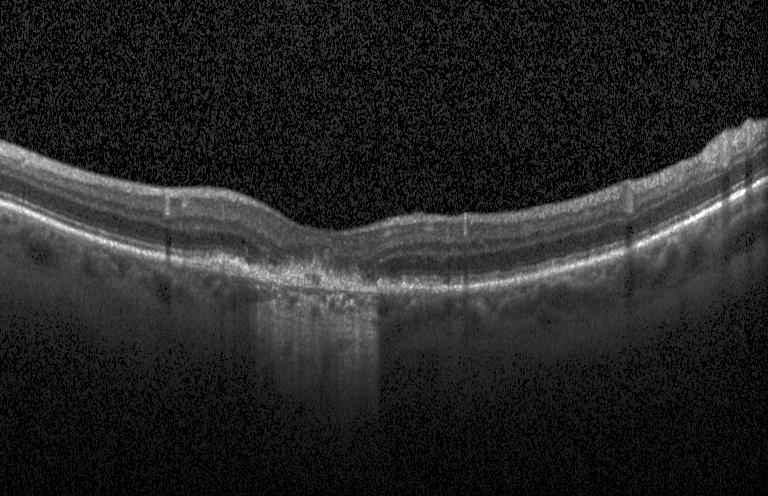 Diagnosis: a choroidal neovascular membrane.